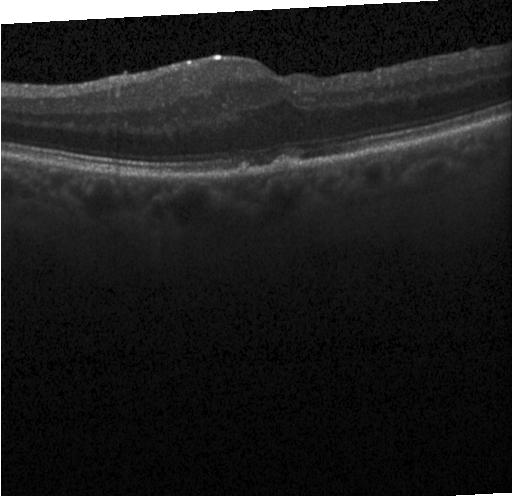

Diagnosis: multiple drusen.